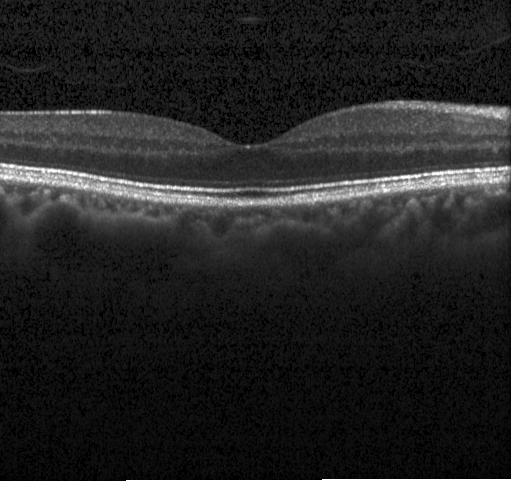

Diagnosis: no evidence of choroidal neovascularization, diabetic macular edema, or drusen.